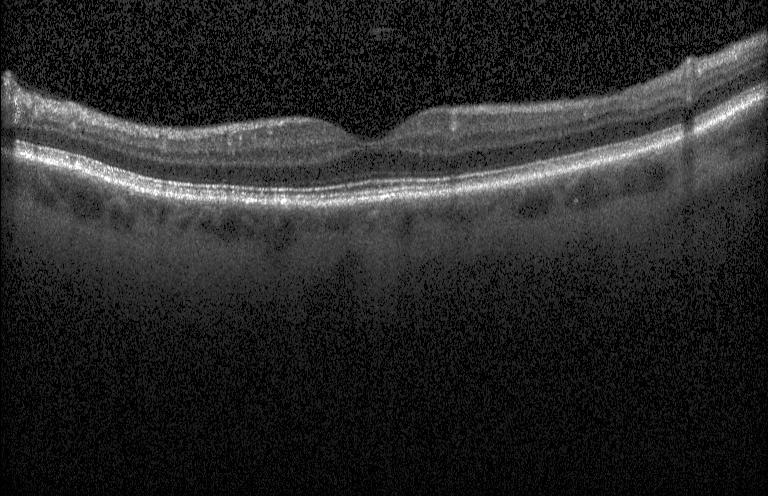
Dx: neither CNV, DME, nor drusen.